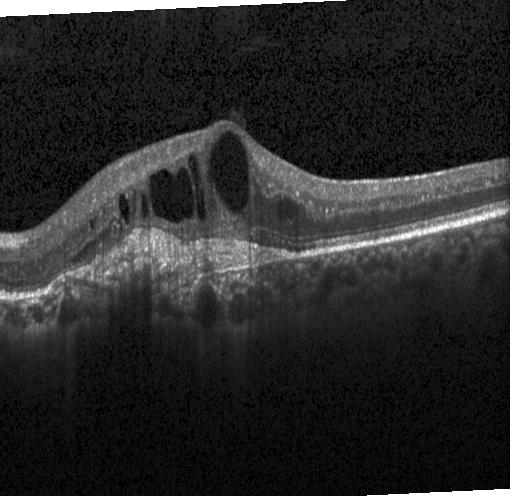
Optical coherence tomography scan — This B-scan demonstrates choroidal neovascularization.